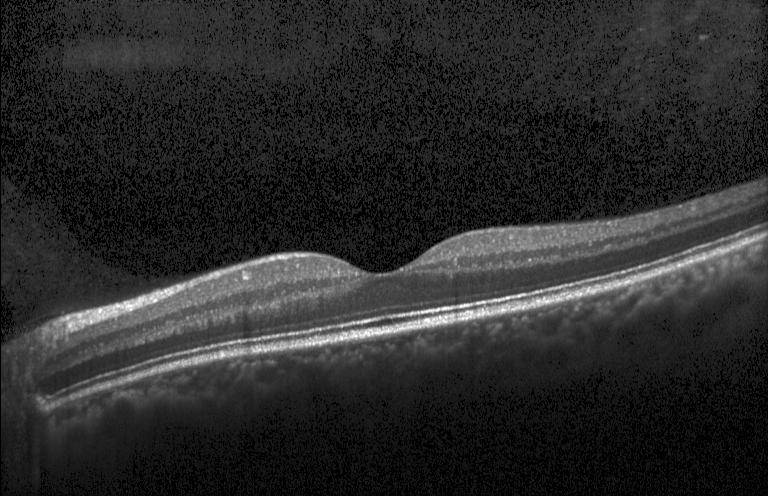 Assessment: neither choroidal neovascularization, diabetic macular edema, nor drusen.